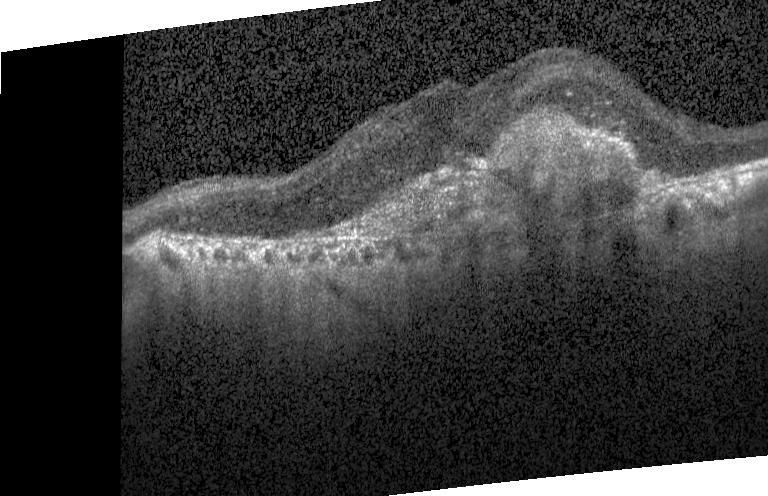

Macular OCT: choroidal neovascularization.